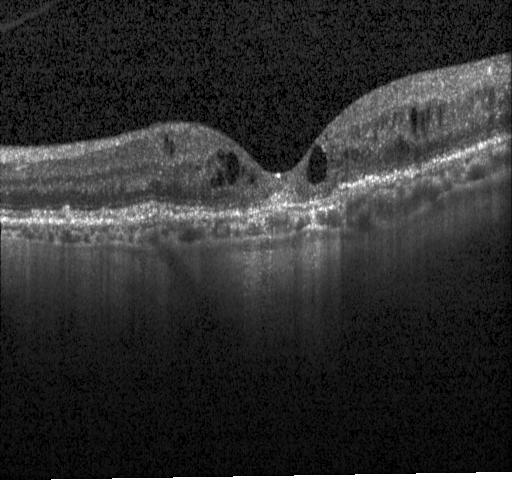
Macular OCT: a choroidal neovascular membrane.